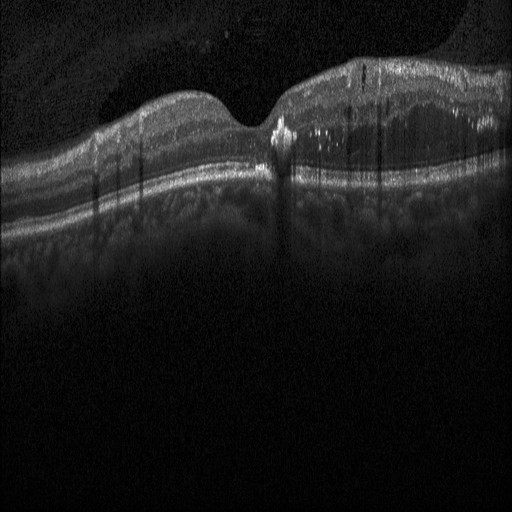

OCT finding: diabetic macular edema.